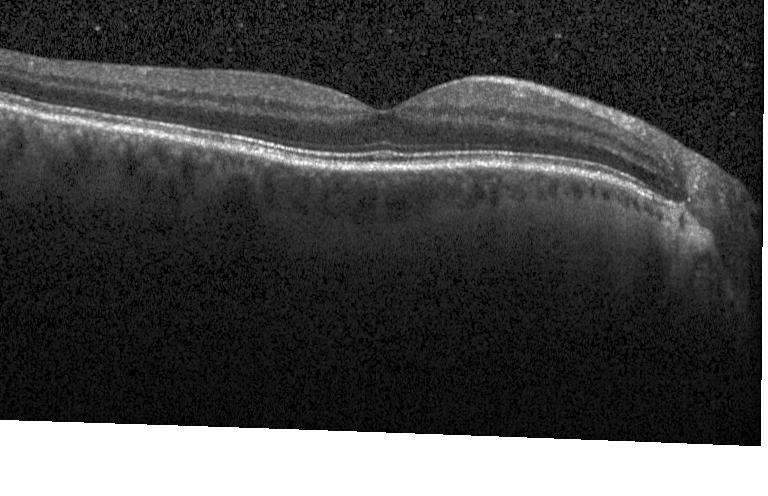
OCT line scan · instrument: Heidelberg Spectralis · SD-OCT
This B-scan demonstrates no choroidal neovascularization, no diabetic macular edema, and no drusen.